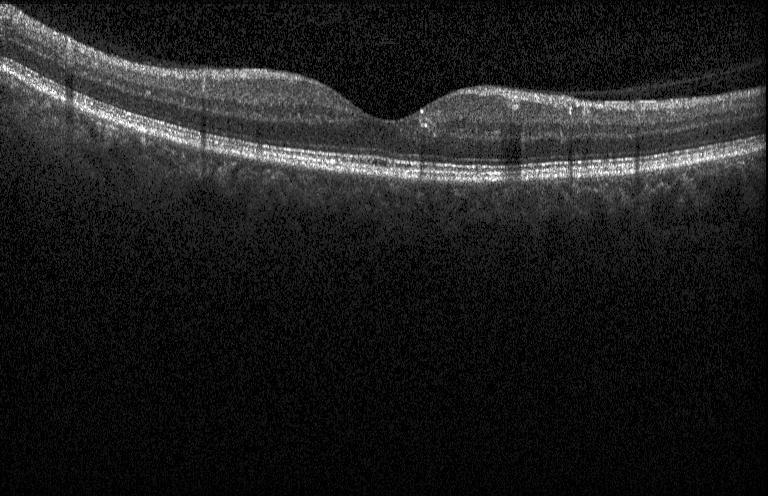
Finding: no choroidal neovascularization, no diabetic macular edema, and no drusen.